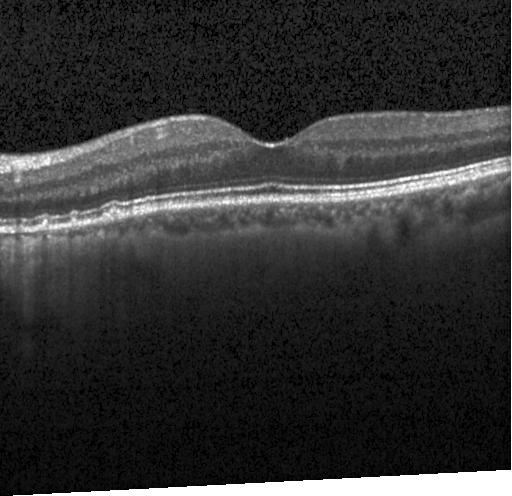

Acquired on a Heidelberg Spectralis. Optical coherence tomography B-scan. SD-OCT. Centered on the fovea.
OCT finding: drusen.